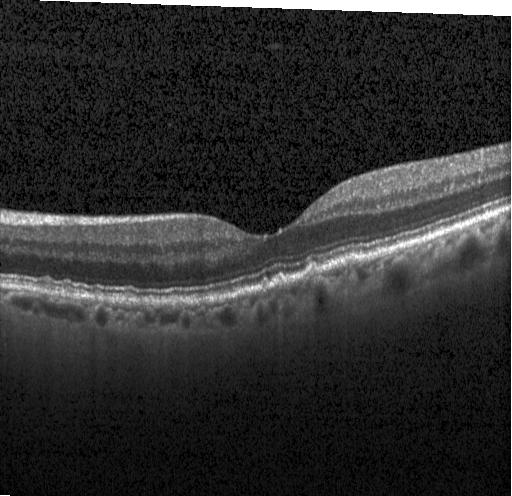 Macular OCT demonstrating multiple drusen.